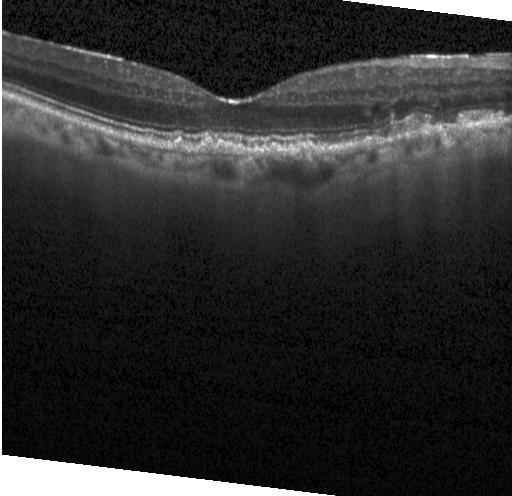

OCT scan showing multiple drusen.